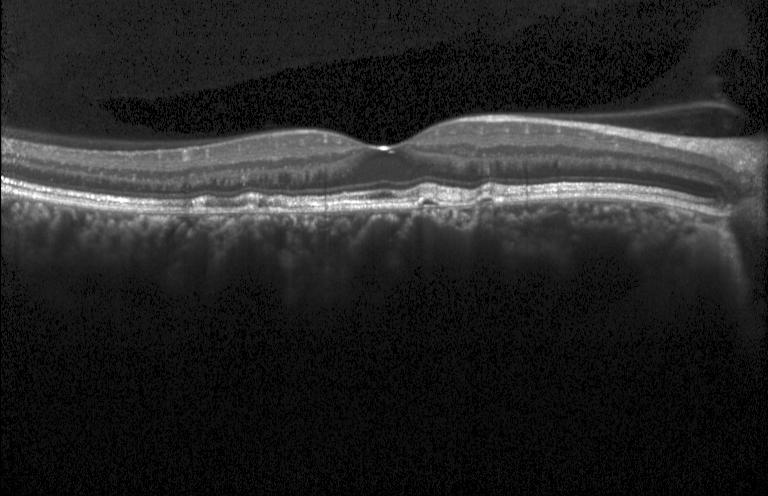 Heidelberg Spectralis, spectral-domain OCT, OCT line scan, fovea-centered — Dx: multiple drusen.